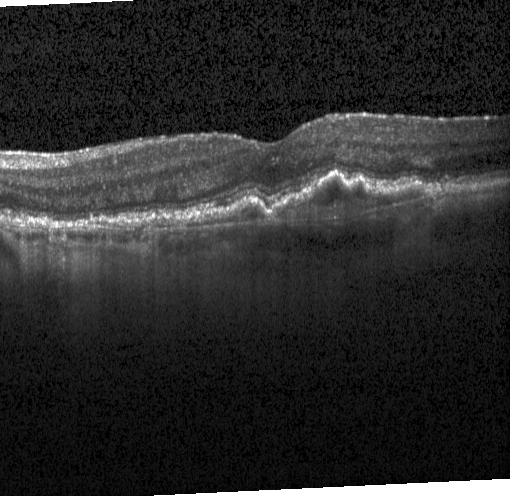
OCT scan showing a choroidal neovascular membrane.